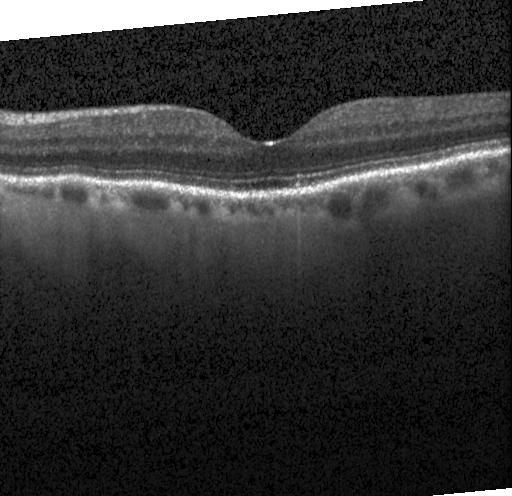
Retinal OCT B-scan
The scan shows no CNV, no DME, and no drusen.